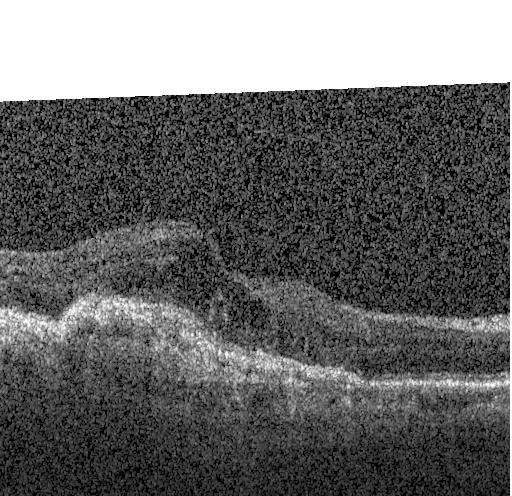
Optical coherence tomography B-scan. Diagnosis: choroidal neovascularization (CNV).